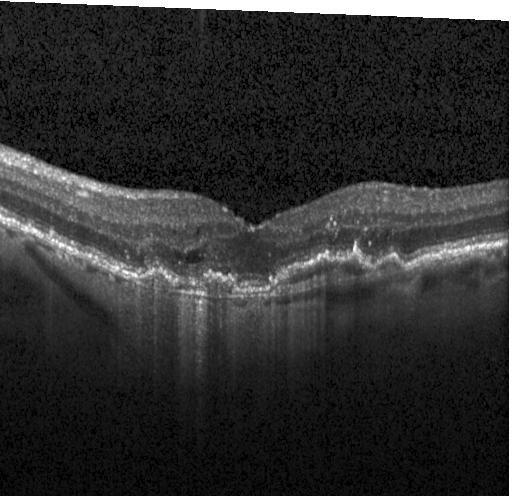
OCT B-scan; acquired on a Heidelberg Spectralis
This B-scan demonstrates choroidal neovascularization (CNV).